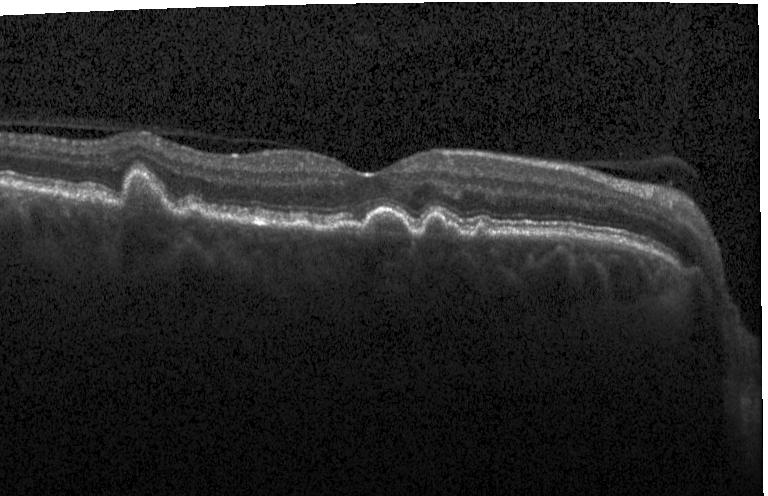

Heidelberg Spectralis OCT system, through the macula, optical coherence tomography B-scan. This B-scan demonstrates drusen.